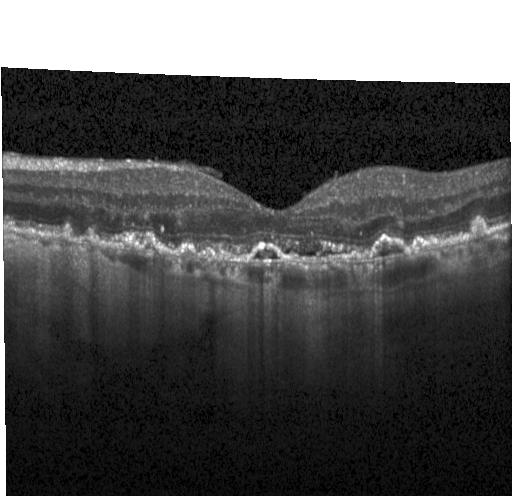

Diagnosis: choroidal neovascularization (CNV).